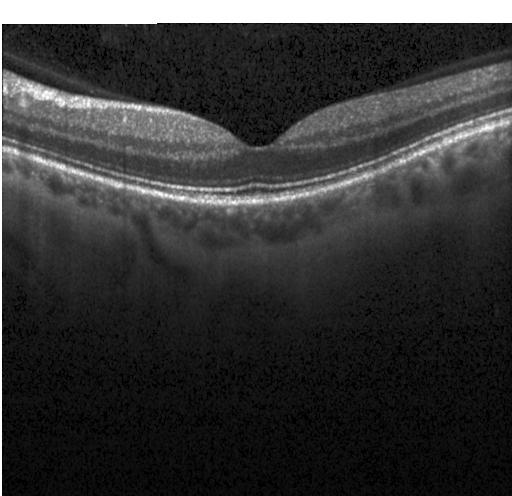 Retinal OCT cross-section · Heidelberg Spectralis. Finding: neither choroidal neovascularization, diabetic macular edema, nor drusen.